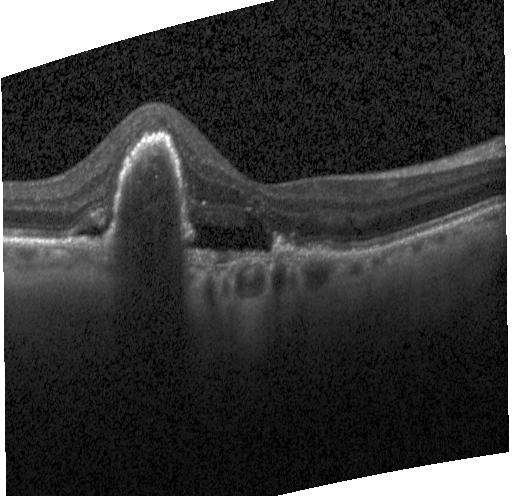 OCT line scan — Dx: a choroidal neovascular membrane.